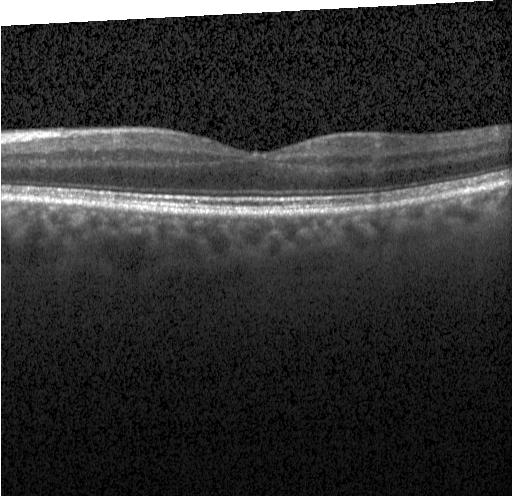

Finding: no choroidal neovascularization, no diabetic macular edema, and no drusen.